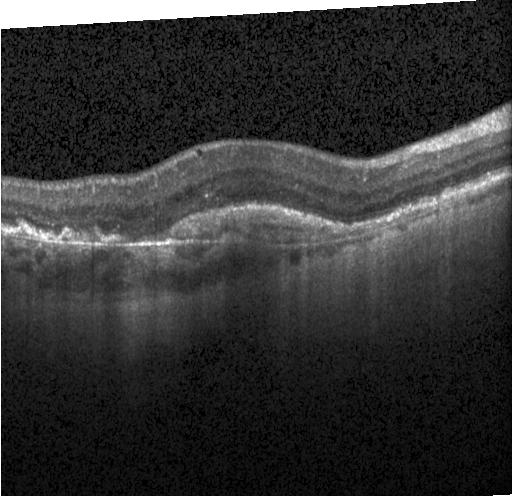
Instrument: Heidelberg Spectralis, optical coherence tomography B-scan. Impression: choroidal neovascularization (CNV).